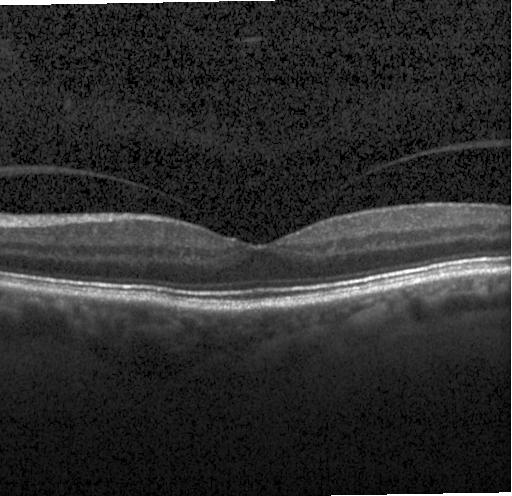 SD-OCT. Heidelberg Spectralis OCT system. OCT B-scan
Diagnosis: no evidence of choroidal neovascularization, diabetic macular edema, or drusen.